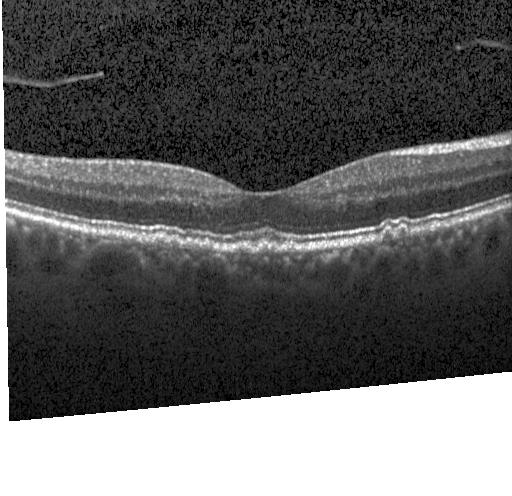 OCT line scan. Finding: sub-RPE drusenoid deposits.